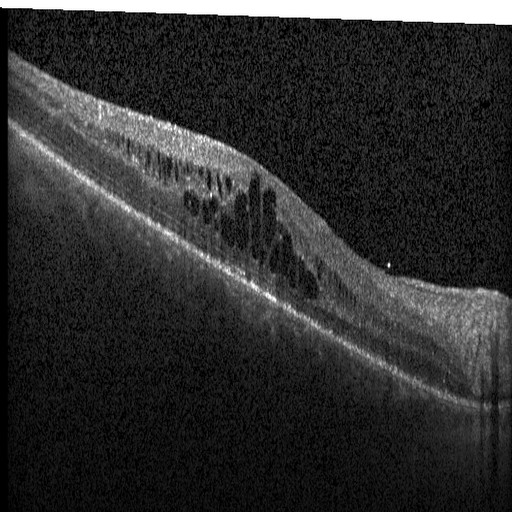

OCT line scan. Centered on the fovea. Heidelberg Spectralis — Dx: DME.